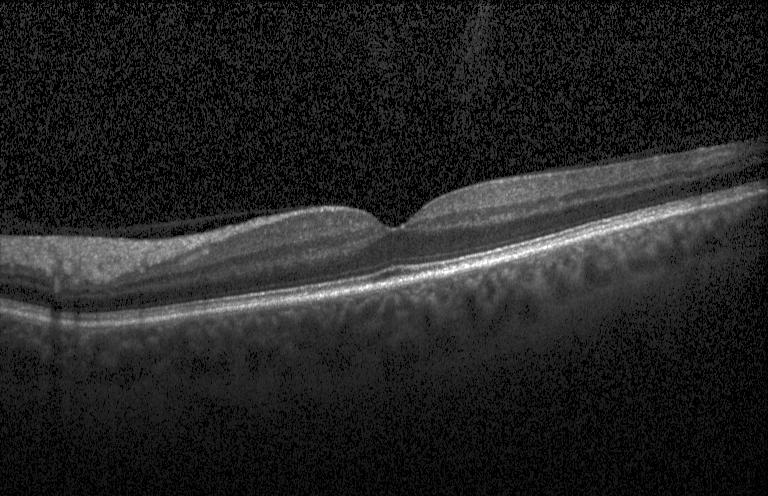
Diagnosis: no choroidal neovascularization, no diabetic macular edema, and no drusen.